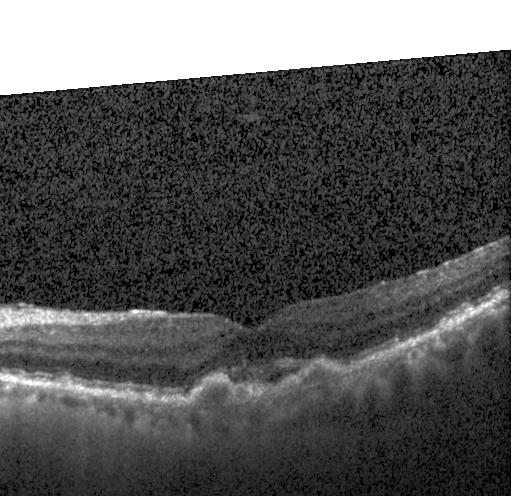 Retinal OCT B-scan, instrument: Heidelberg Spectralis, spectral-domain optical coherence tomography, macular scan.
Diagnosis: a choroidal neovascular membrane.